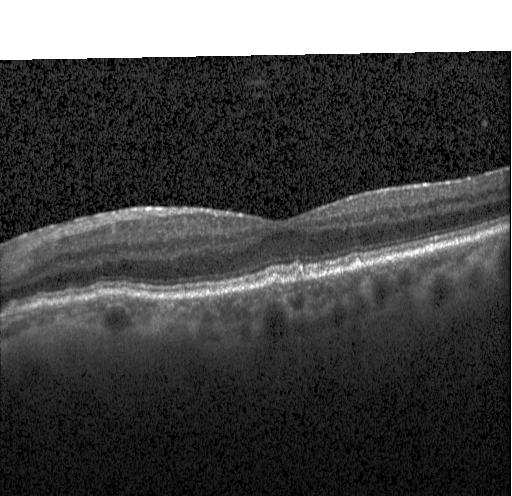

Retinal OCT B-scan; centered on the fovea; instrument: Heidelberg Spectralis; spectral-domain optical coherence tomography — Macular OCT: drusen.